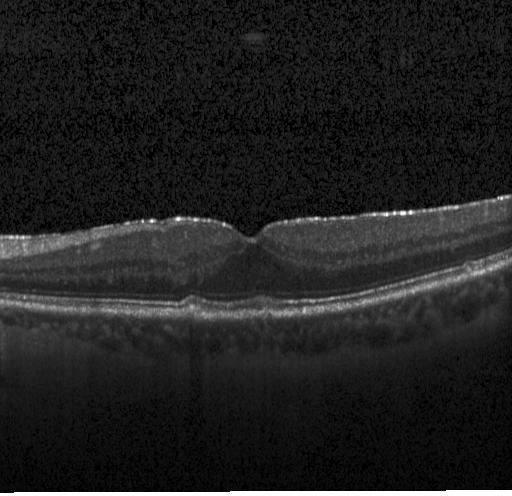
OCT scan showing multiple drusen.